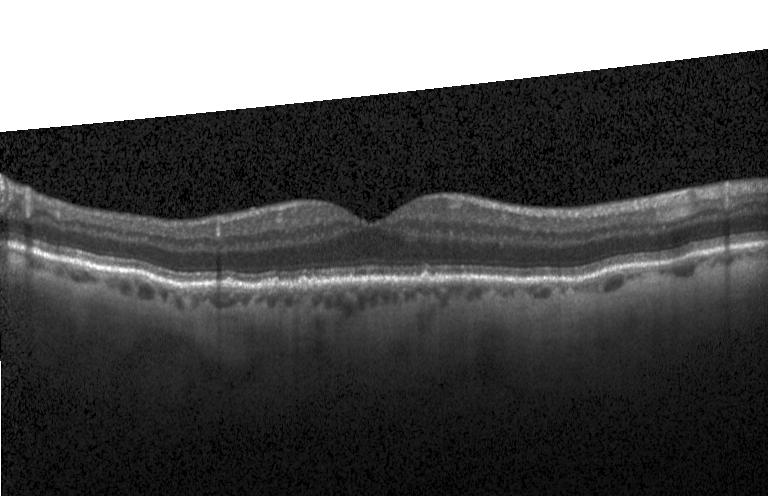 OCT scan showing multiple drusen.